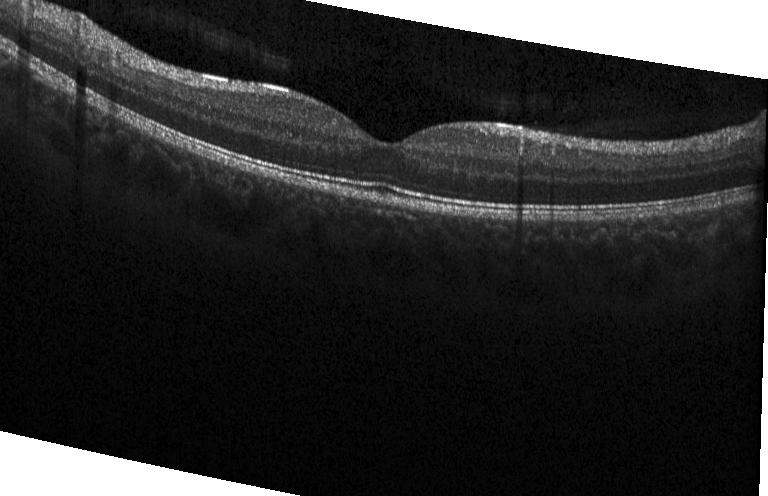
Macular OCT: no evidence of CNV, DME, or drusen.